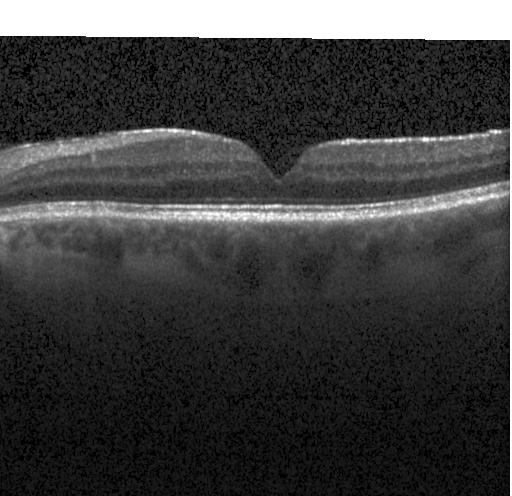

No evidence of choroidal neovascularization, diabetic macular edema, or drusen.